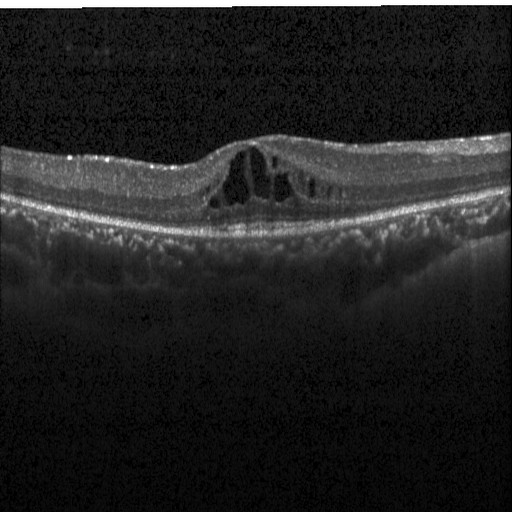
Optical coherence tomography B-scan. Macular OCT: DME.